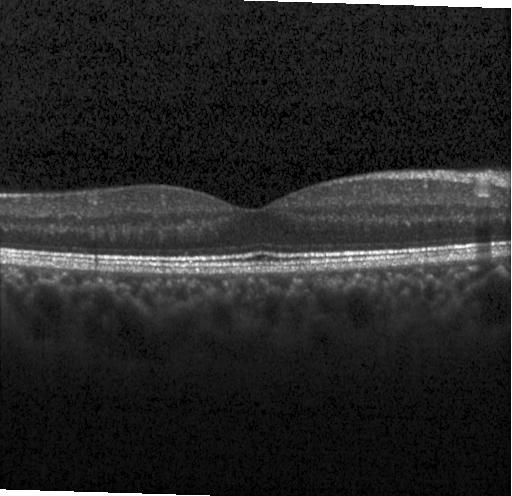

Centered on the fovea, retinal OCT B-scan. Diagnosis: no evidence of choroidal neovascularization, diabetic macular edema, or drusen.